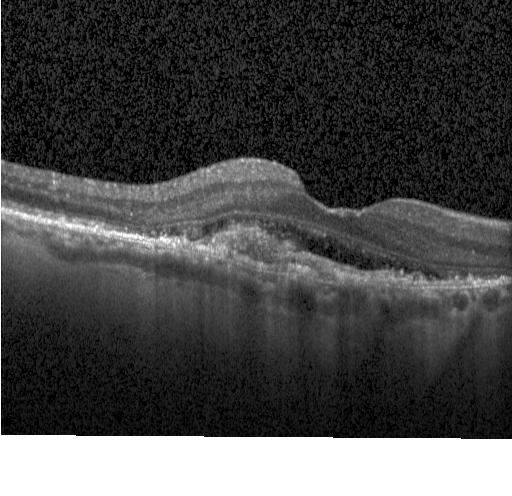 Optical coherence tomography B-scan; Heidelberg Spectralis OCT system; fovea-centered; spectral-domain optical coherence tomography
Assessment: CNV.